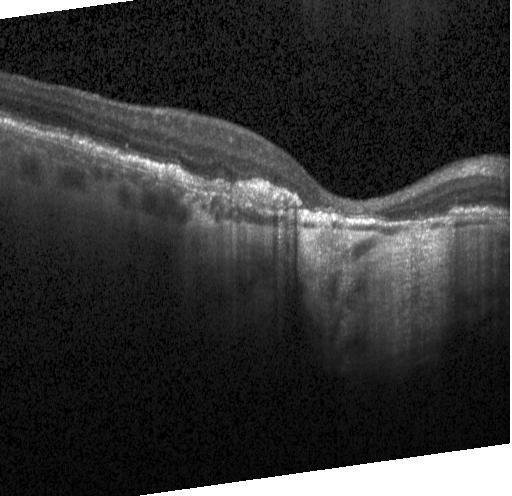

Optical coherence tomography B-scan
Diagnosis: a choroidal neovascular membrane.